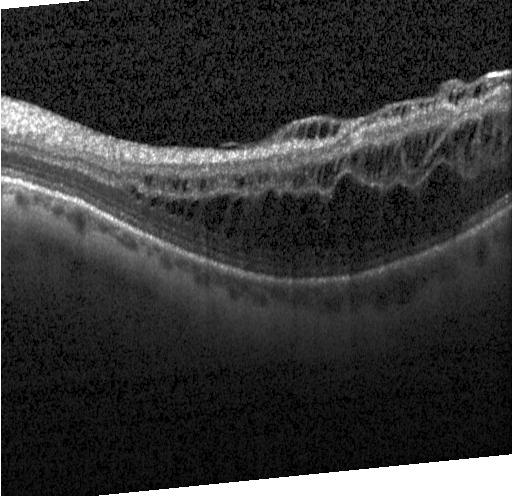 Instrument: Heidelberg Spectralis · OCT line scan · macular scan — Finding: diabetic macular edema (DME).